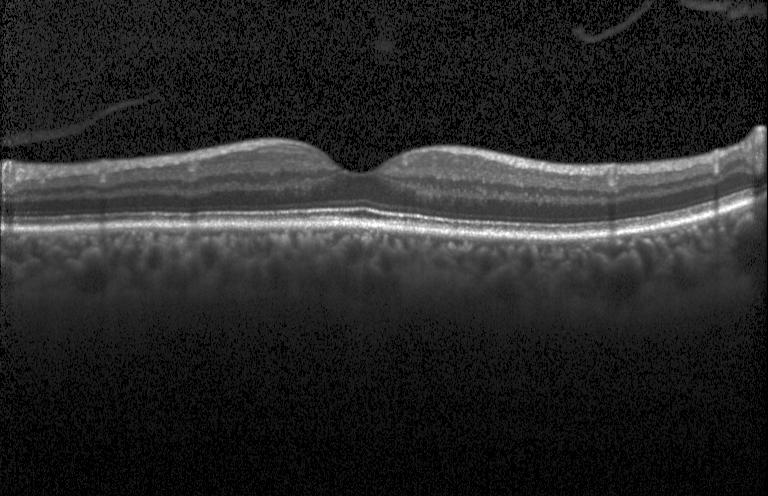

Retinal OCT B-scan. Macular OCT: neither choroidal neovascularization, diabetic macular edema, nor drusen.